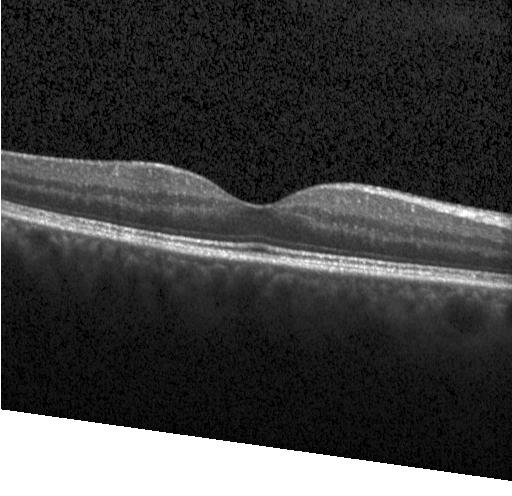

Instrument: Heidelberg Spectralis; optical coherence tomography scan; spectral-domain OCT; centered on the fovea
The scan shows neither choroidal neovascularization, diabetic macular edema, nor drusen.